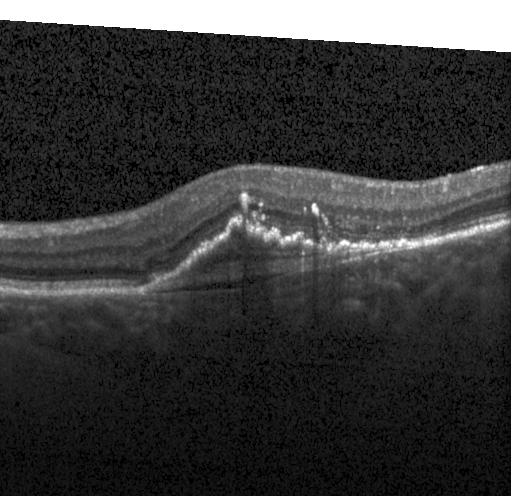

Optical coherence tomography scan. Impression: choroidal neovascularization (CNV).